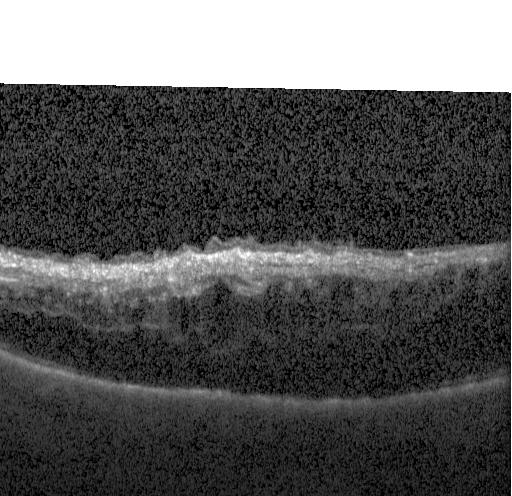 Retinal OCT cross-section
Dx: diabetic macular edema.